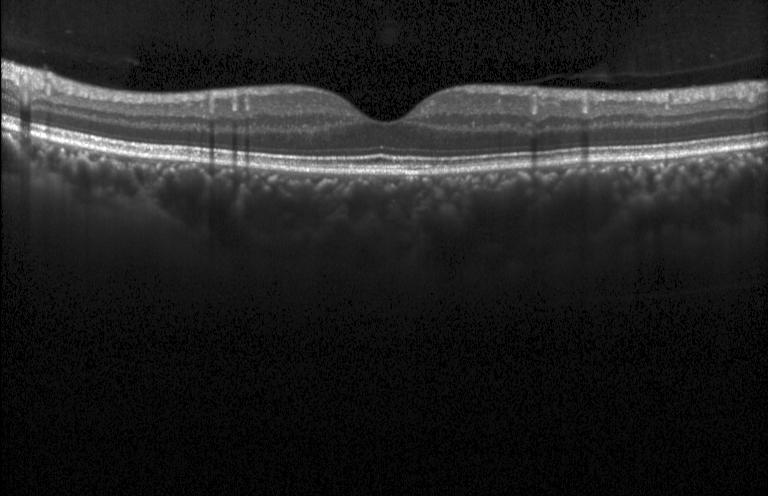
Spectral-domain OCT, optical coherence tomography B-scan.
Diagnosis: no evidence of choroidal neovascularization, diabetic macular edema, or drusen.